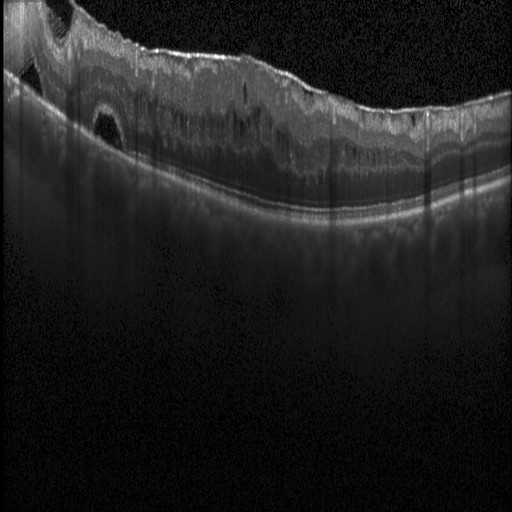 Macular scan; retinal OCT B-scan; instrument: Heidelberg Spectralis; SD-OCT
Diagnosis: DME.